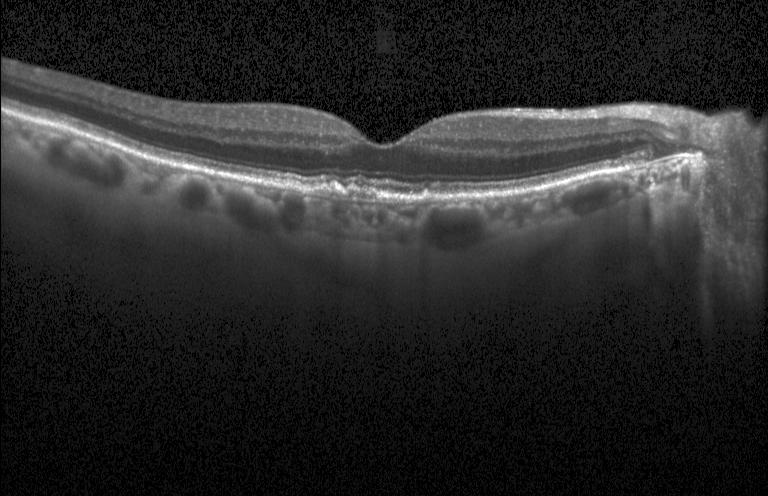 Macular OCT demonstrating sub-RPE drusenoid deposits.